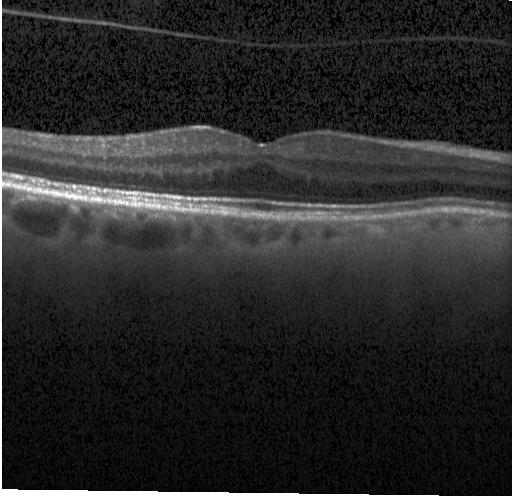

SD-OCT; retinal OCT cross-section.
This B-scan demonstrates no choroidal neovascularization, diabetic macular edema, or drusen.